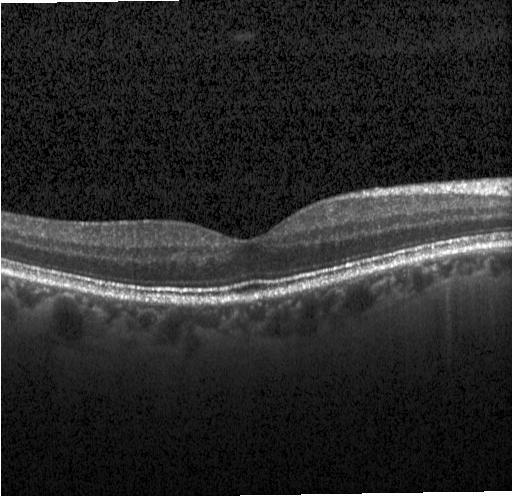 Impression: no choroidal neovascularization, no diabetic macular edema, and no drusen.